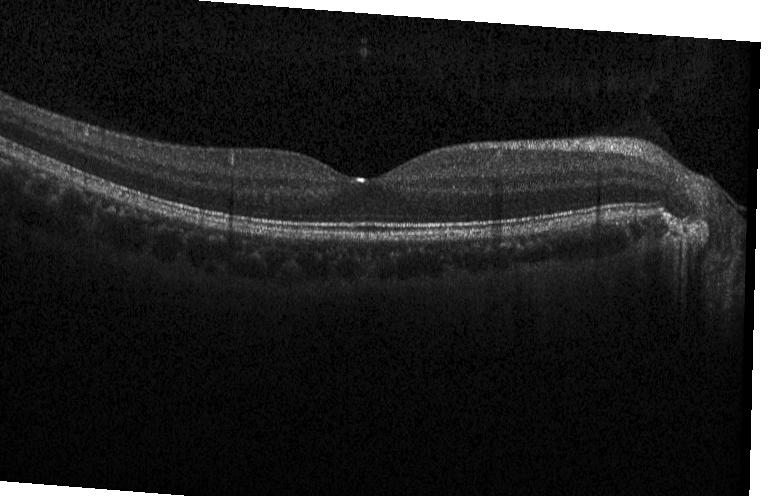

OCT B-scan; instrument: Heidelberg Spectralis; SD-OCT; macular scan
Assessment: neither CNV, DME, nor drusen.